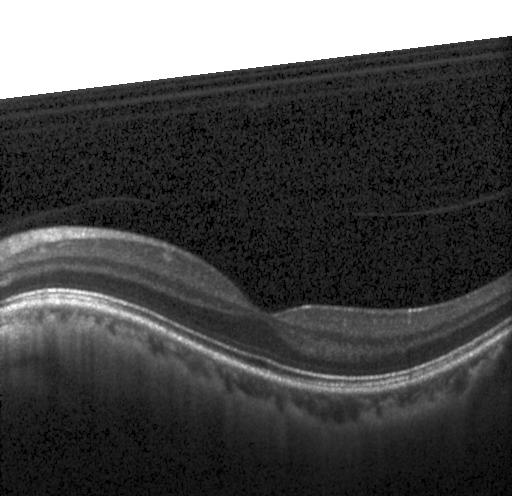
Retinal OCT B-scan
Assessment: no evidence of choroidal neovascularization, diabetic macular edema, or drusen.